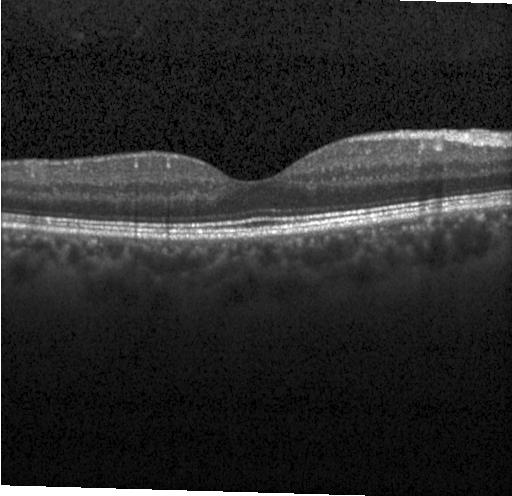

Optical coherence tomography B-scan · fovea-centered · SD-OCT · Heidelberg Spectralis OCT system
Finding: no choroidal neovascularization, diabetic macular edema, or drusen.